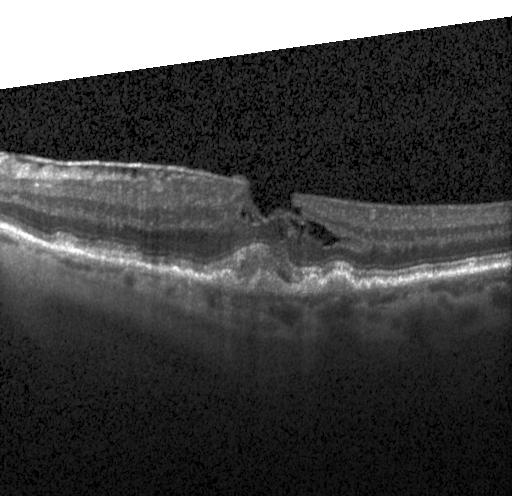
OCT B-scan showing a choroidal neovascular membrane.